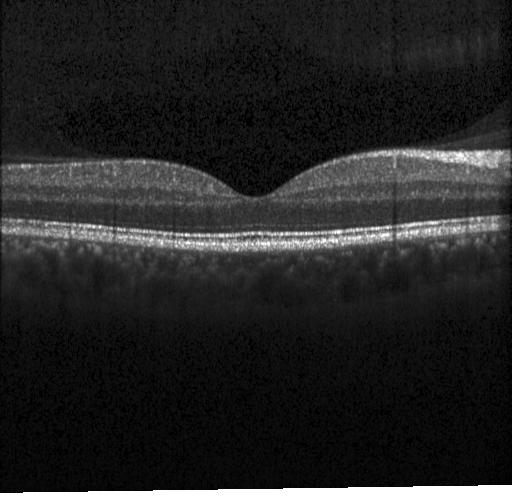 Assessment: neither CNV, DME, nor drusen.